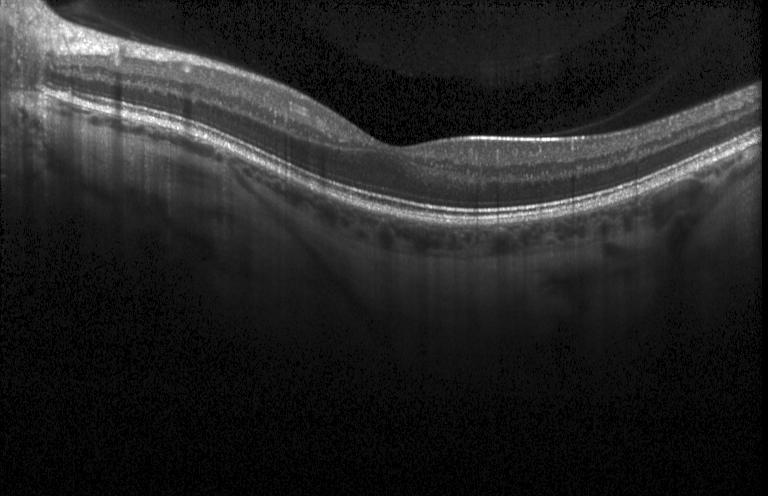 Spectral-domain OCT B-scan: no CNV, no DME, and no drusen.